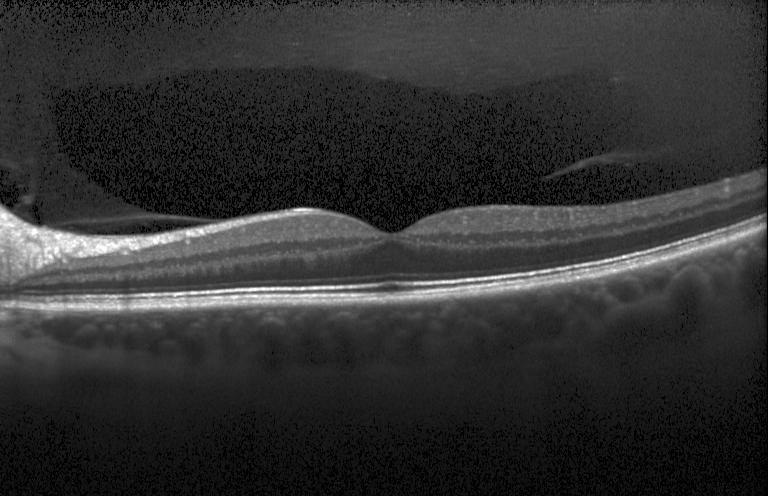 OCT line scan
Diagnosis: no choroidal neovascularization, no diabetic macular edema, and no drusen.